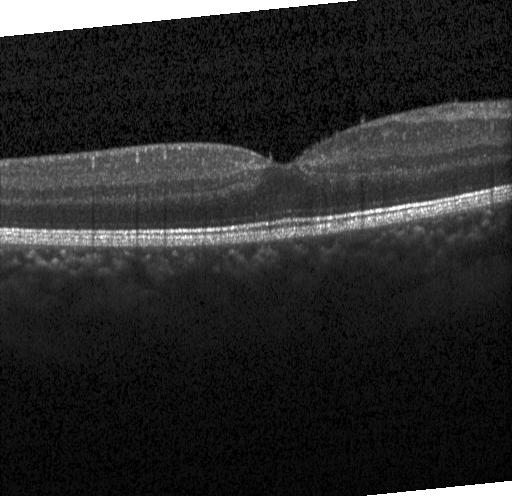
Optical coherence tomography scan · spectral-domain OCT — Diagnosis: neither choroidal neovascularization, diabetic macular edema, nor drusen.